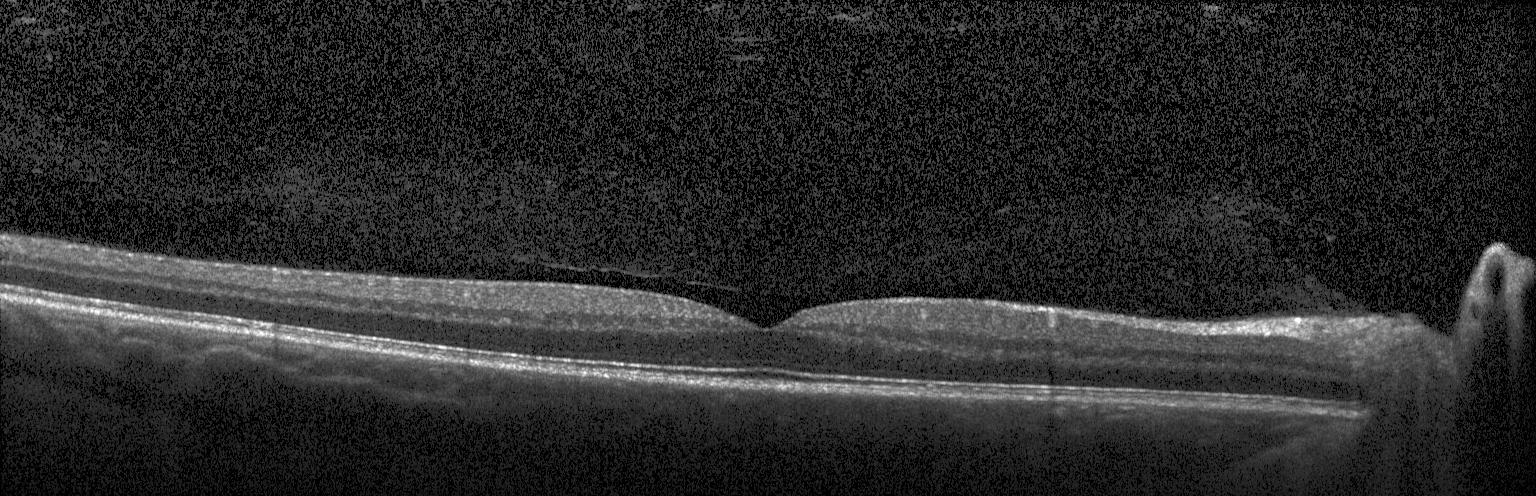

Heidelberg Spectralis; OCT line scan; SD-OCT.
OCT finding: no evidence of CNV, DME, or drusen.